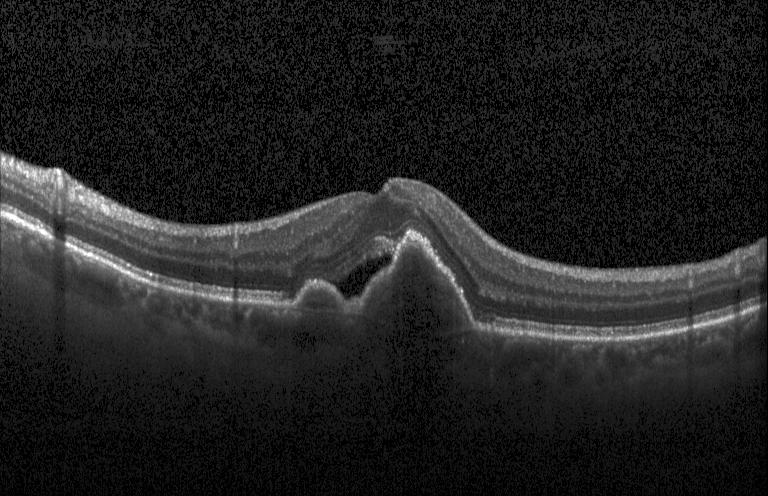

Macular scan, instrument: Heidelberg Spectralis, SD-OCT, retinal OCT cross-section.
The scan shows choroidal neovascularization (CNV).